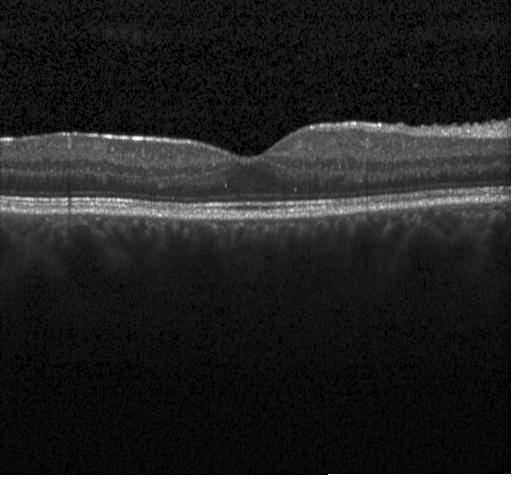

Fovea-centered · OCT line scan · Heidelberg Spectralis · spectral-domain optical coherence tomography
Finding: neither choroidal neovascularization, diabetic macular edema, nor drusen.